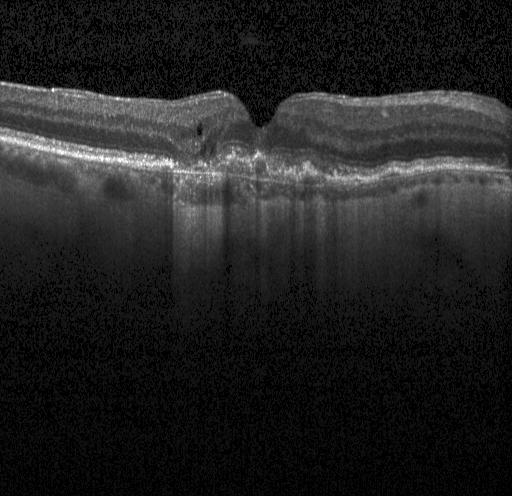

Spectral-domain OCT B-scan: CNV.